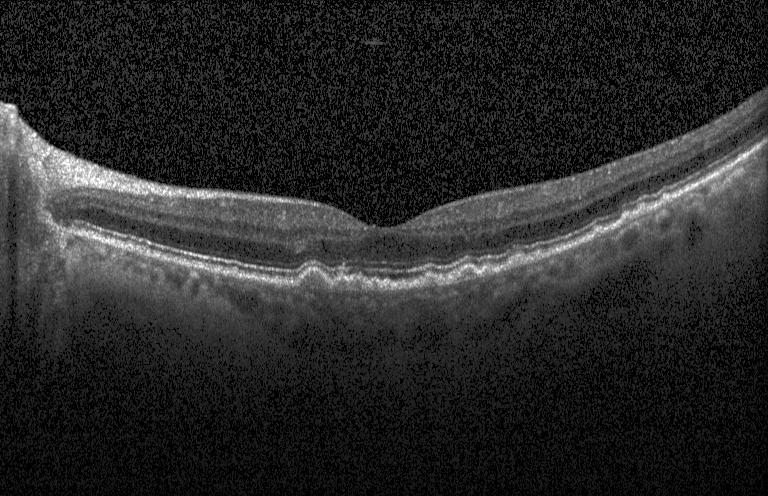
Retinal OCT cross-section. OCT finding: multiple drusen.